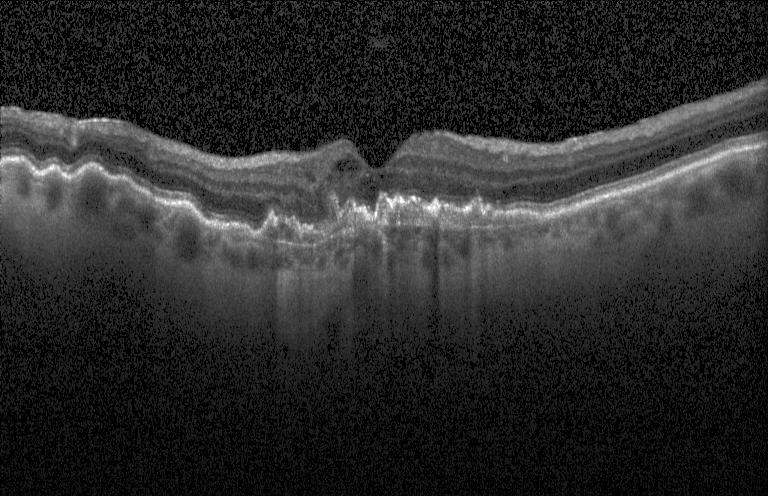 Retinal OCT cross-section showing choroidal neovascularization (CNV).